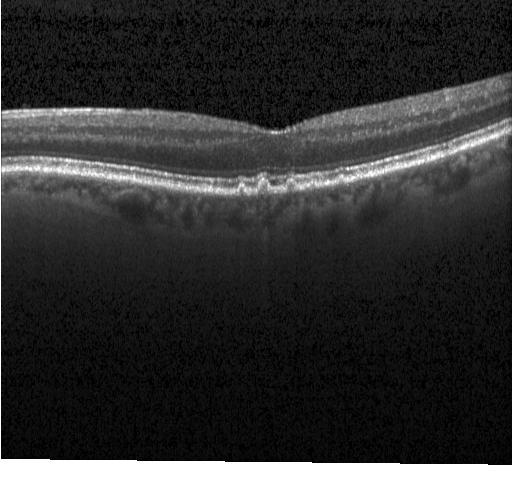

OCT B-scan showing drusen.